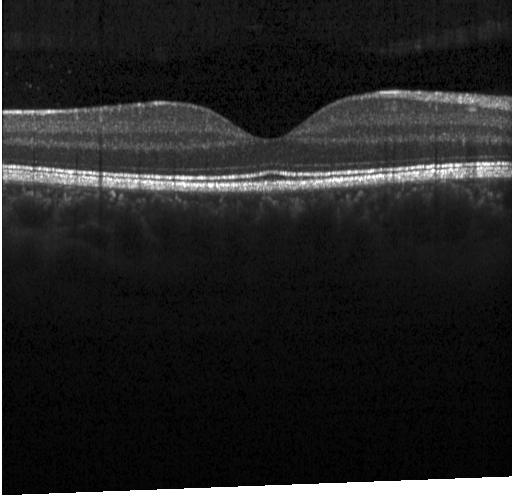

Horizontal scan through the fovea · OCT B-scan · spectral-domain optical coherence tomography — Impression: no choroidal neovascularization, diabetic macular edema, or drusen.